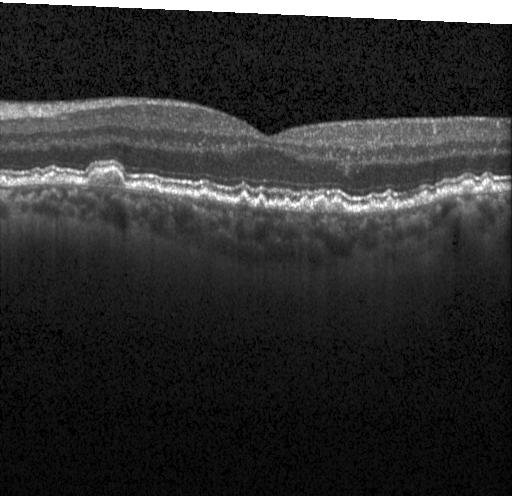 Optical coherence tomography scan; Heidelberg Spectralis OCT system.
Assessment: drusen.